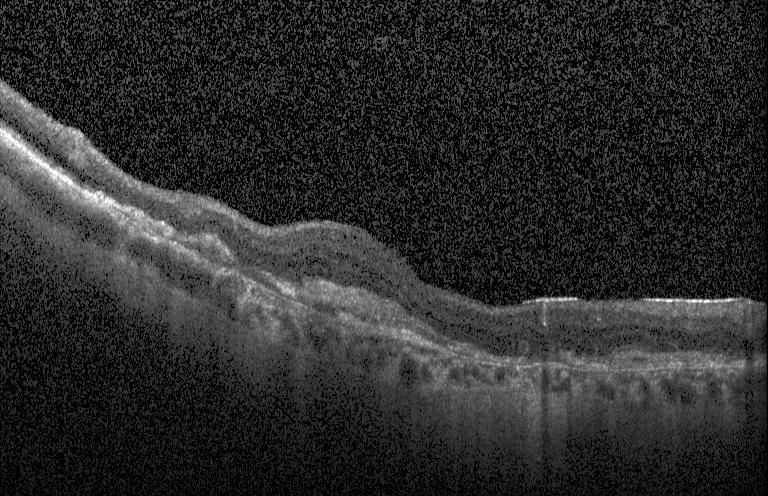 Optical coherence tomography scan
A choroidal neovascular membrane.